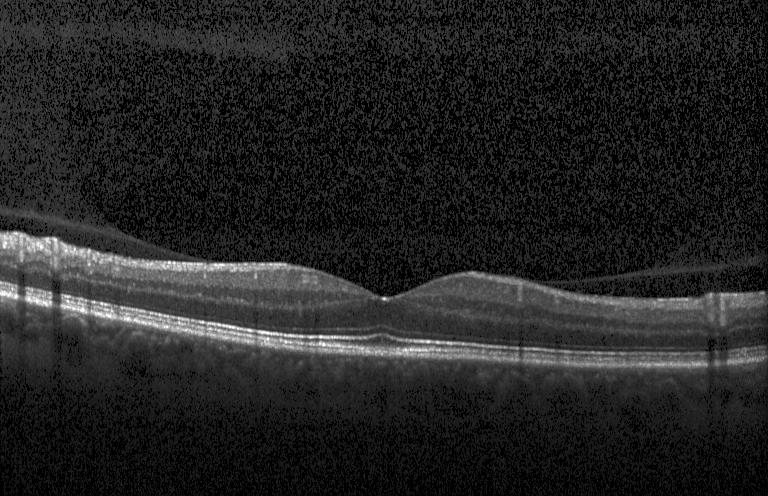 Optical coherence tomography B-scan. Diagnosis: no choroidal neovascularization, no diabetic macular edema, and no drusen.